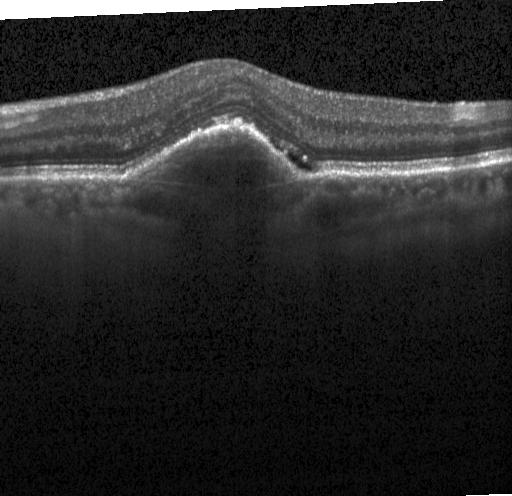
Diagnosis: a choroidal neovascular membrane.